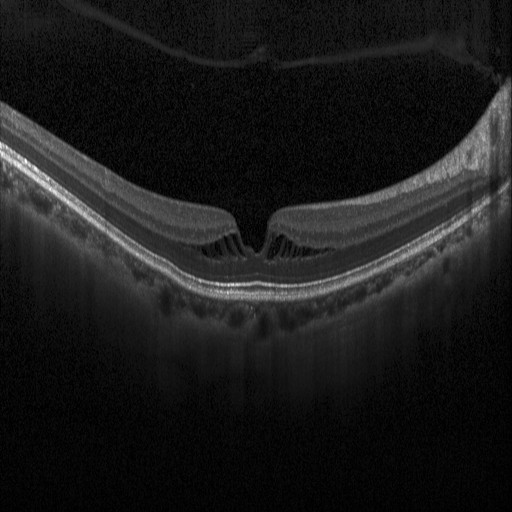 SD-OCT. Through the macula. Optical coherence tomography scan. Instrument: Heidelberg Spectralis.
Impression: diabetic macular edema.